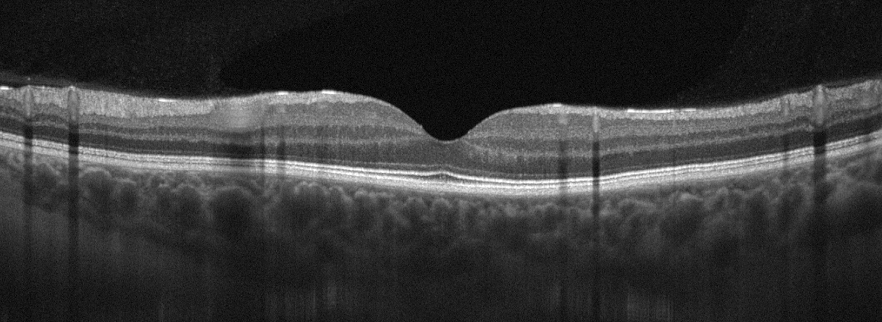 Optical coherence tomography scan. Macular scan. Acquired on an Optovue Avanti RTVue XR.
Impression: no AMD, DME, ERM, RAO, RVO, or VID.